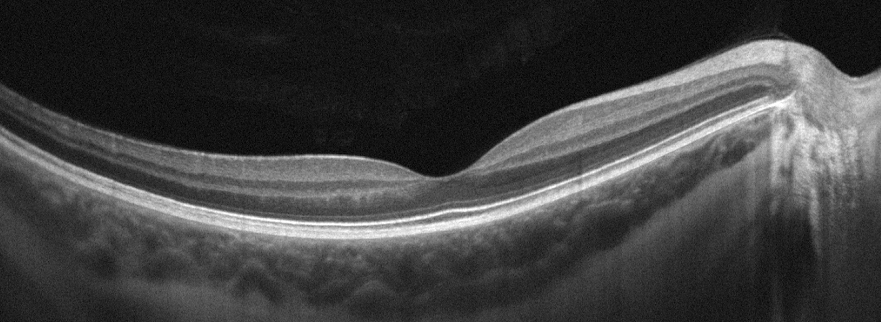 Right eye; Optovue Avanti RTVue XR; through the macula; retinal OCT B-scan — The scan shows no evidence of AMD, DME, ERM, RAO, RVO, or VID.